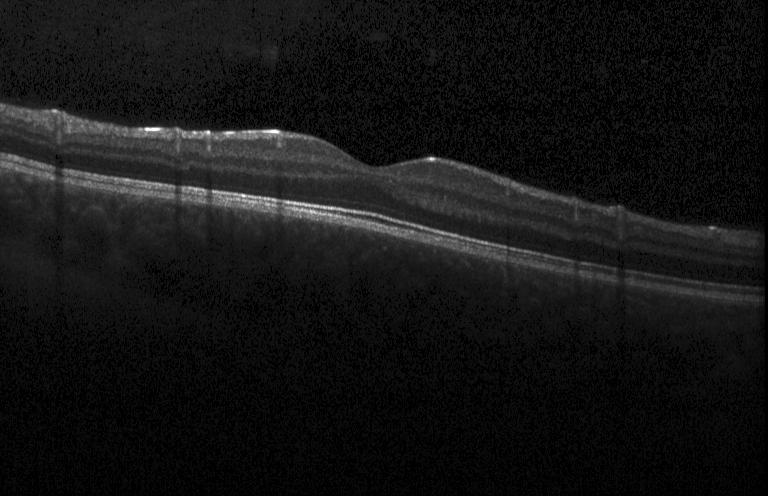
Through the macula. Spectral-domain OCT. Acquired on a Heidelberg Spectralis. Retinal OCT B-scan
Diagnosis: no evidence of choroidal neovascularization, diabetic macular edema, or drusen.